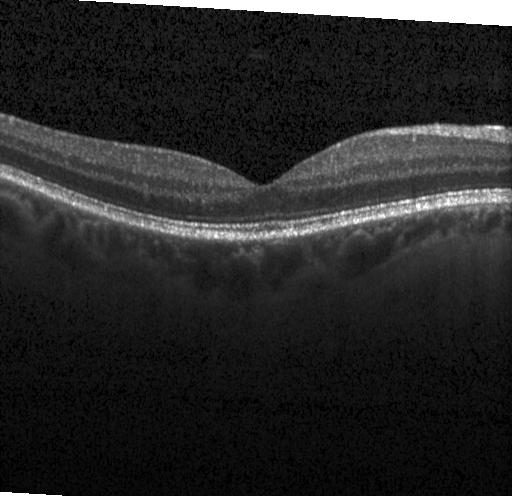

Fovea-centered, retinal OCT B-scan, instrument: Heidelberg Spectralis, SD-OCT — This B-scan demonstrates no evidence of choroidal neovascularization, diabetic macular edema, or drusen.